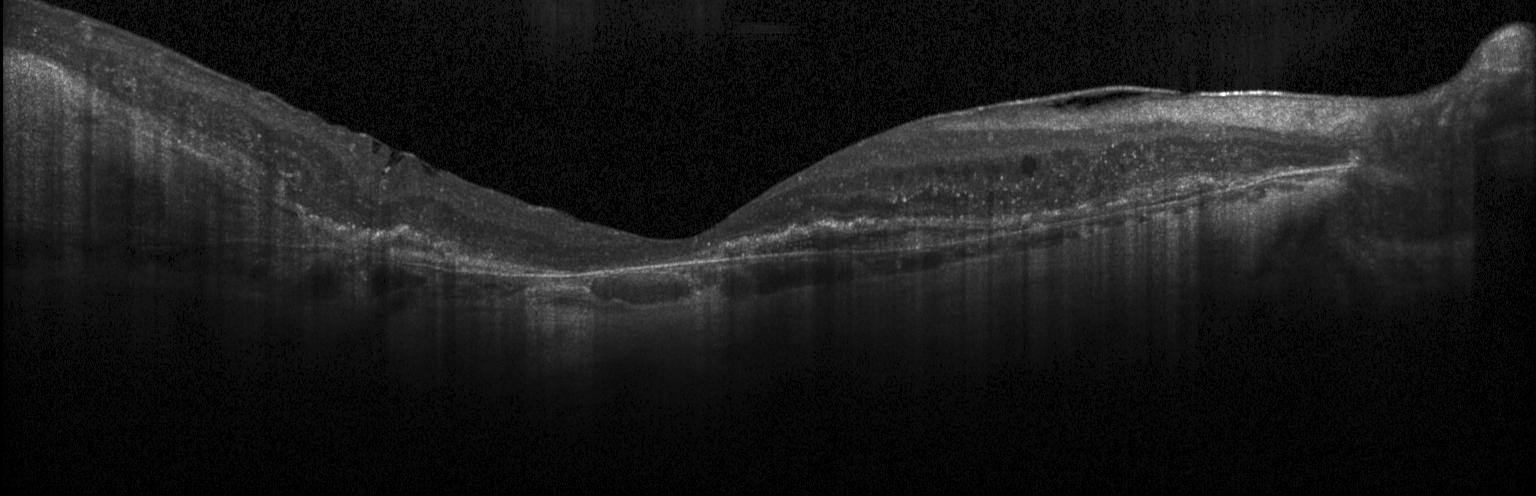
Impression: a choroidal neovascular membrane.